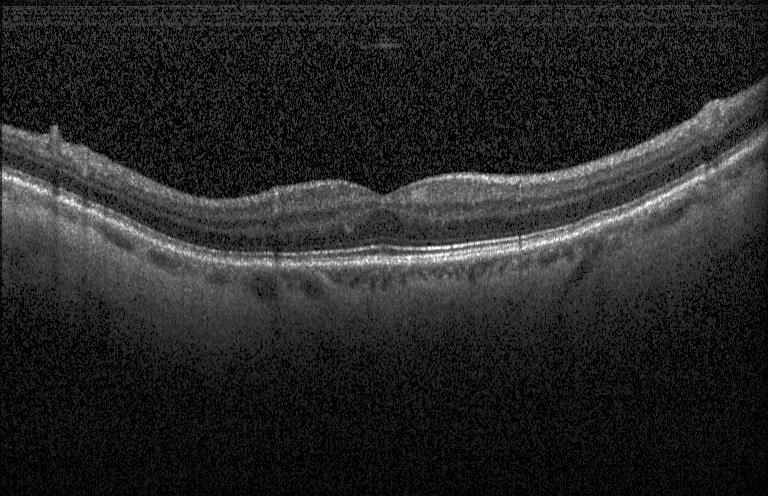 Dx: neither CNV, DME, nor drusen.